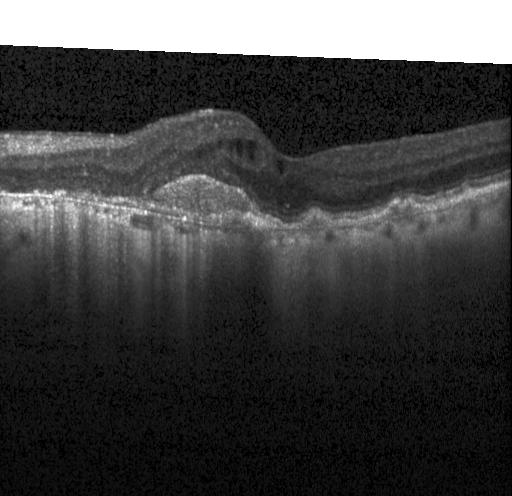

Spectral-domain OCT, through the macula, optical coherence tomography B-scan. The scan shows a choroidal neovascular membrane.